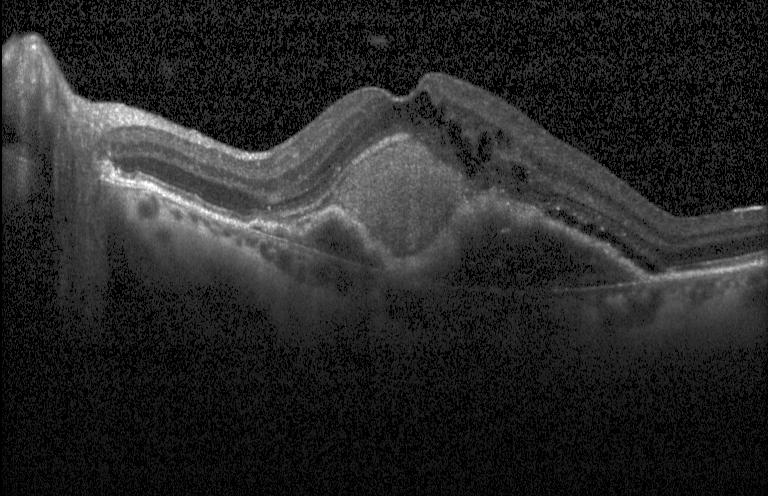 Spectral-domain OCT, OCT B-scan — This B-scan demonstrates CNV.